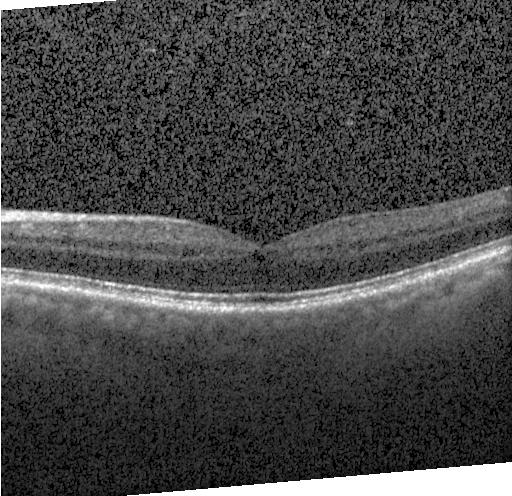 Finding: no choroidal neovascularization, no diabetic macular edema, and no drusen.